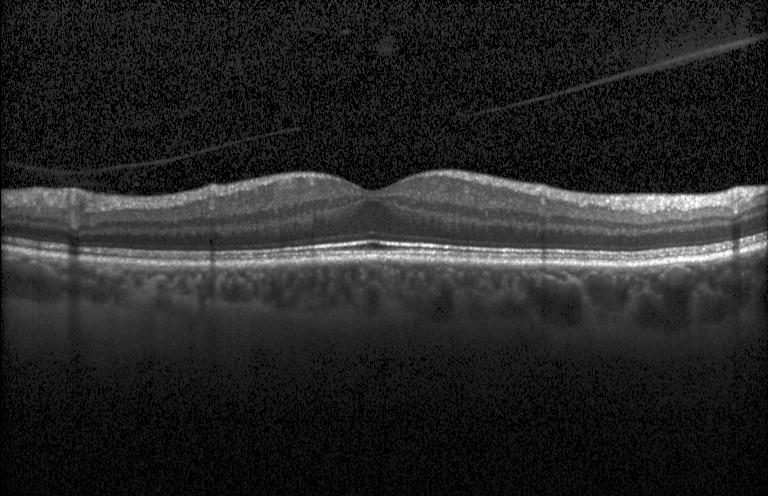

This B-scan demonstrates no CNV, no DME, and no drusen.